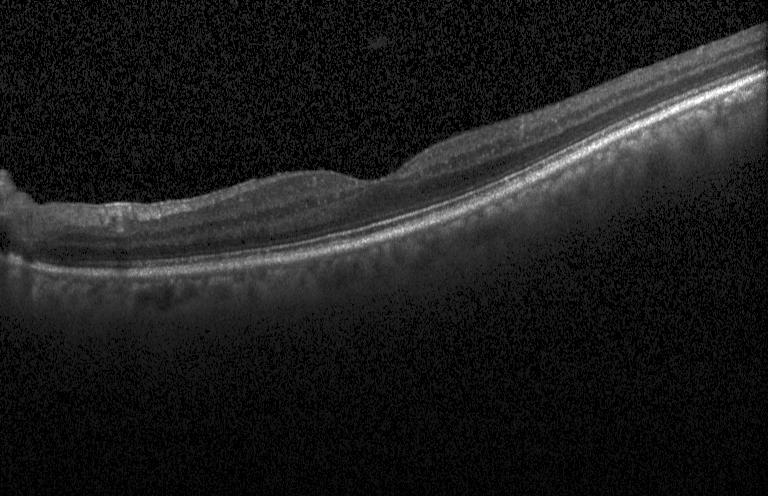

Through the macula, optical coherence tomography scan, instrument: Heidelberg Spectralis, spectral-domain OCT. Assessment: no choroidal neovascularization, no diabetic macular edema, and no drusen.